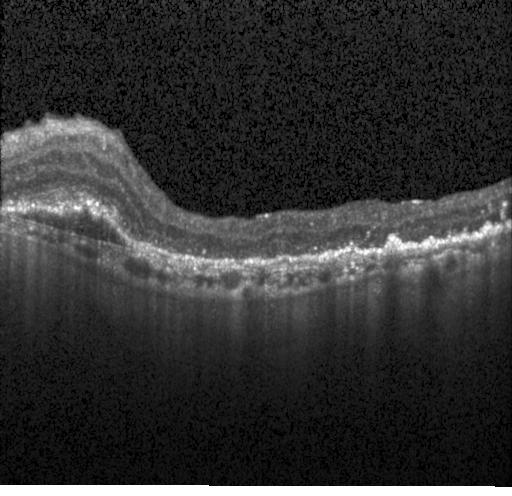
SD-OCT · retinal OCT cross-section — The scan shows a choroidal neovascular membrane.